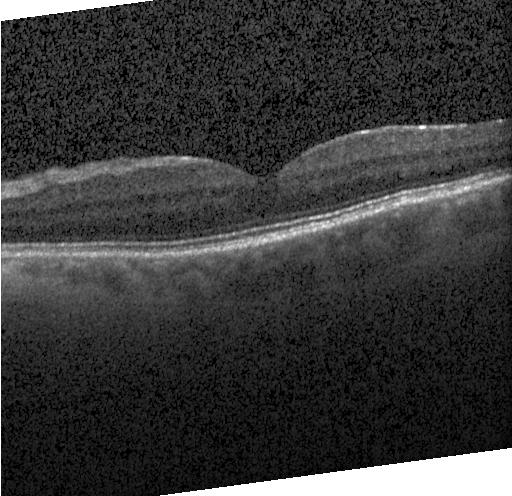
Macular OCT: neither choroidal neovascularization, diabetic macular edema, nor drusen.